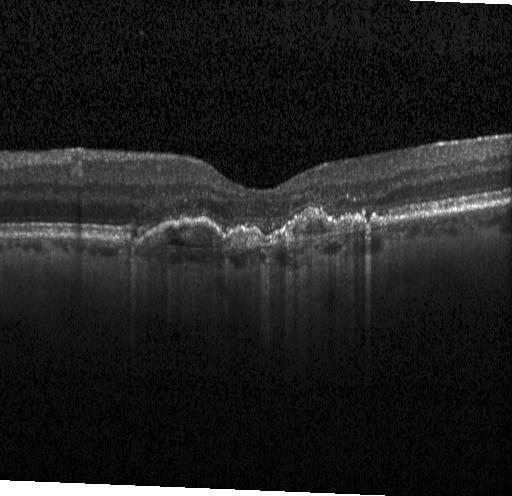 Impression: a choroidal neovascular membrane.